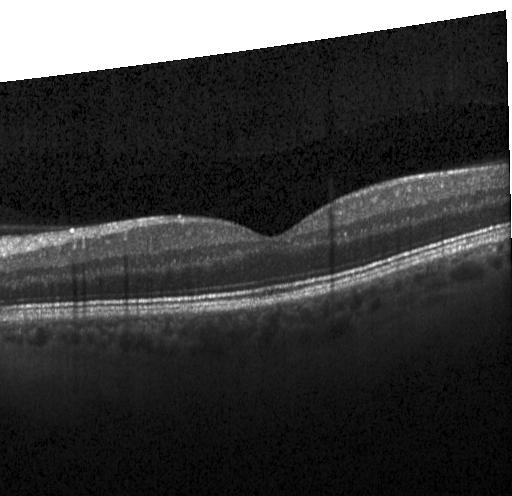
Diagnosis: no evidence of choroidal neovascularization, diabetic macular edema, or drusen.